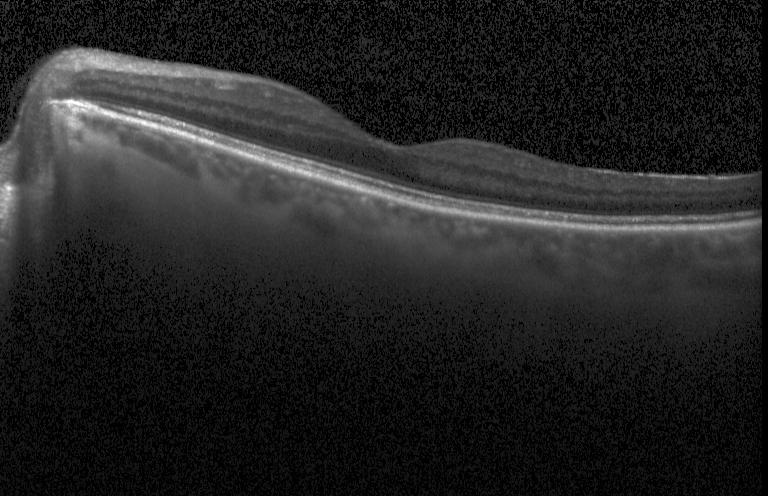
Fovea-centered, optical coherence tomography scan. Dx: no choroidal neovascularization, diabetic macular edema, or drusen.